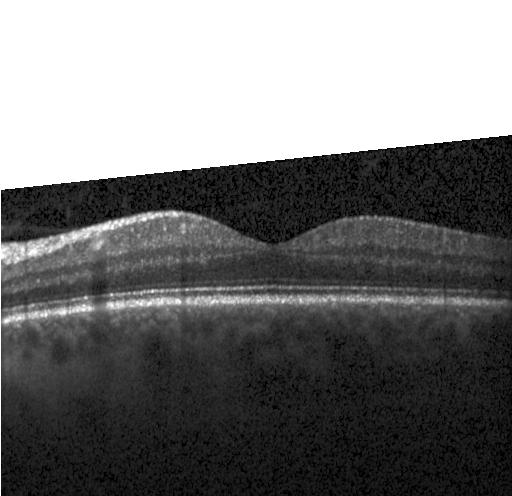 Retinal OCT B-scan — Impression: no choroidal neovascularization, diabetic macular edema, or drusen.